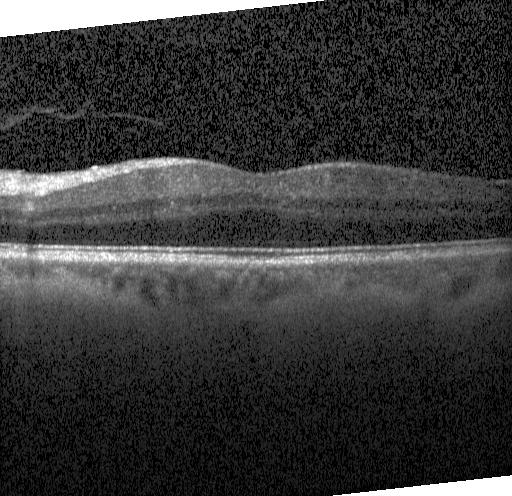 Retinal OCT B-scan, through the macula, Heidelberg Spectralis OCT system, spectral-domain optical coherence tomography.
Finding: neither choroidal neovascularization, diabetic macular edema, nor drusen.